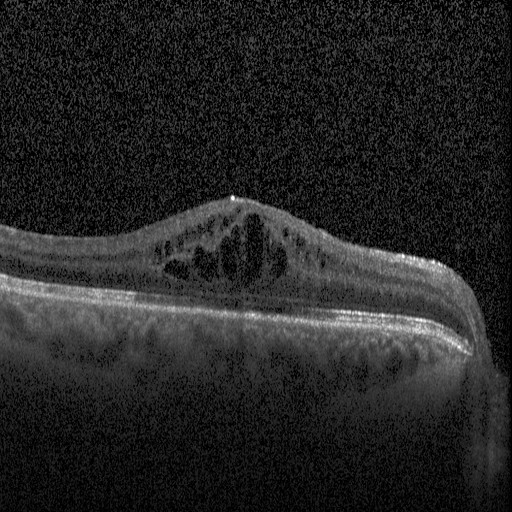

Heidelberg Spectralis OCT system · optical coherence tomography B-scan.
This B-scan demonstrates diabetic macular edema (DME).